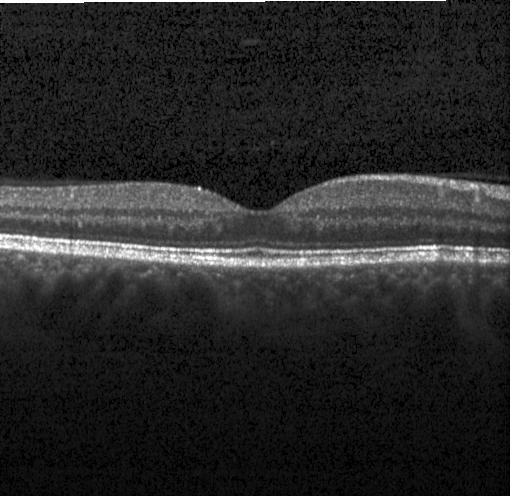 Retinal OCT B-scan, Heidelberg Spectralis OCT system. The scan shows no choroidal neovascularization, diabetic macular edema, or drusen.